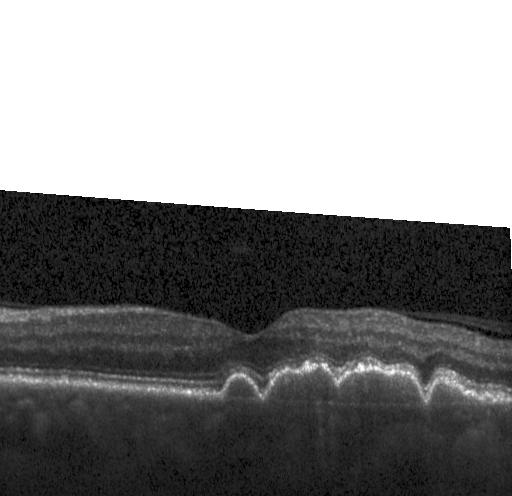 Heidelberg Spectralis OCT system, macular scan, spectral-domain OCT, optical coherence tomography scan. Diagnosis: sub-RPE drusenoid deposits.